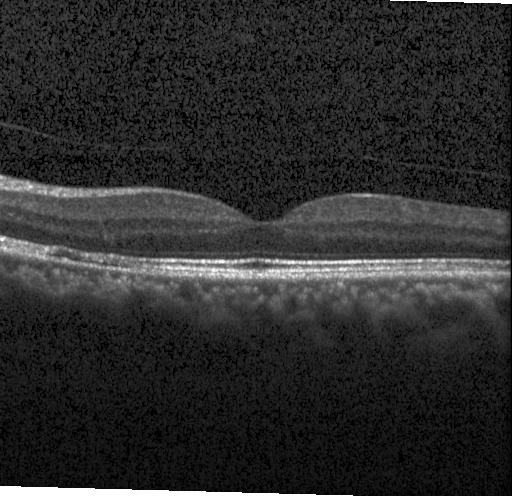

Heidelberg Spectralis; optical coherence tomography scan; macular scan.
Macular OCT: neither choroidal neovascularization, diabetic macular edema, nor drusen.